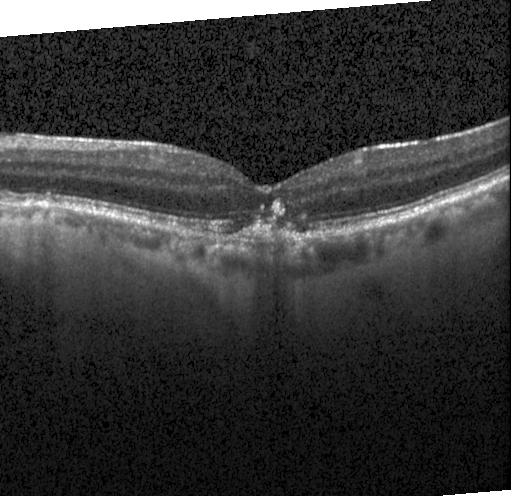
Retinal OCT cross-section showing choroidal neovascularization.